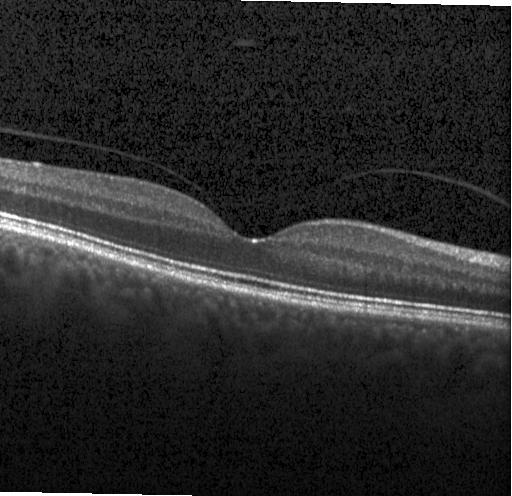 Optical coherence tomography B-scan; spectral-domain OCT; instrument: Heidelberg Spectralis. No CNV, no DME, and no drusen.